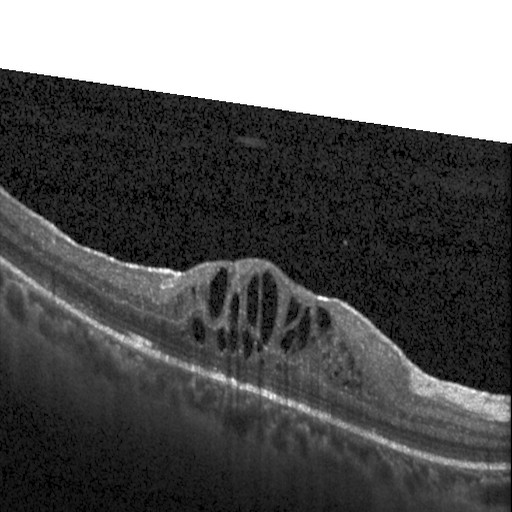 Instrument: Heidelberg Spectralis · optical coherence tomography B-scan · centered on the fovea · spectral-domain optical coherence tomography.
Diagnosis: diabetic macular edema.